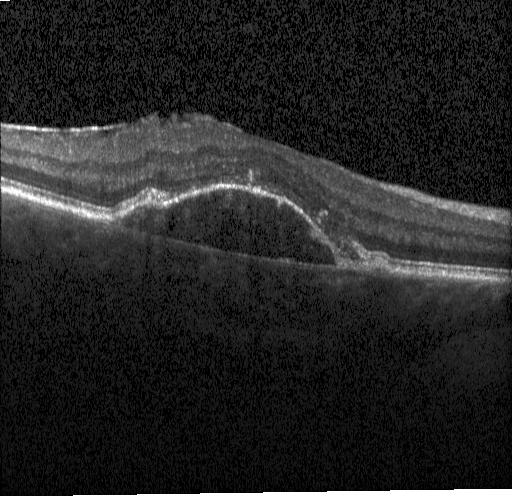 Acquired on a Heidelberg Spectralis. Optical coherence tomography B-scan. Spectral-domain OCT. Through the macula
This B-scan demonstrates a choroidal neovascular membrane.